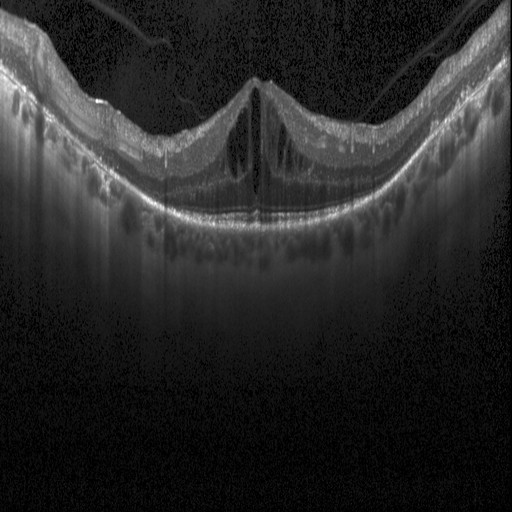 Diagnosis: diabetic macular edema.